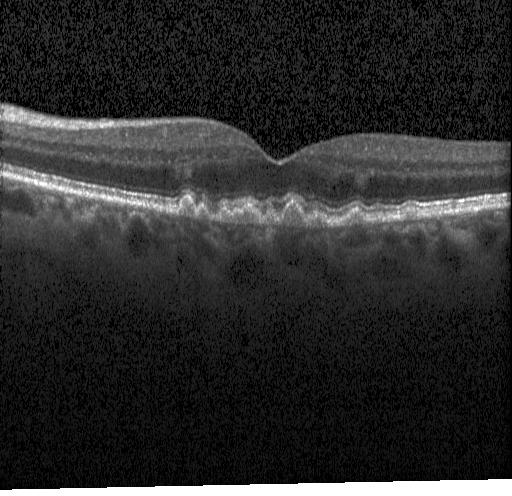
Macular OCT: sub-RPE drusenoid deposits.